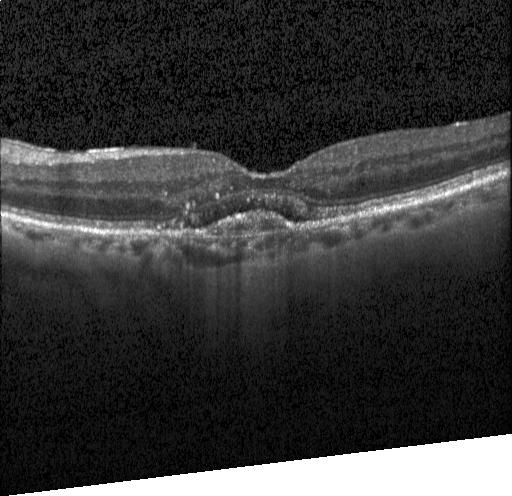
OCT B-scan showing choroidal neovascularization (CNV).